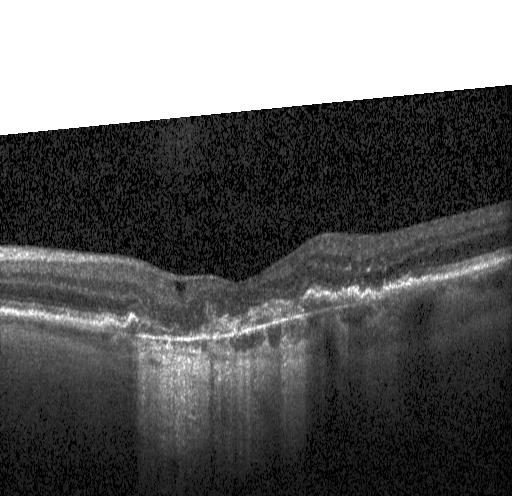 Acquired on a Heidelberg Spectralis. SD-OCT. OCT B-scan
Diagnosis: a choroidal neovascular membrane.